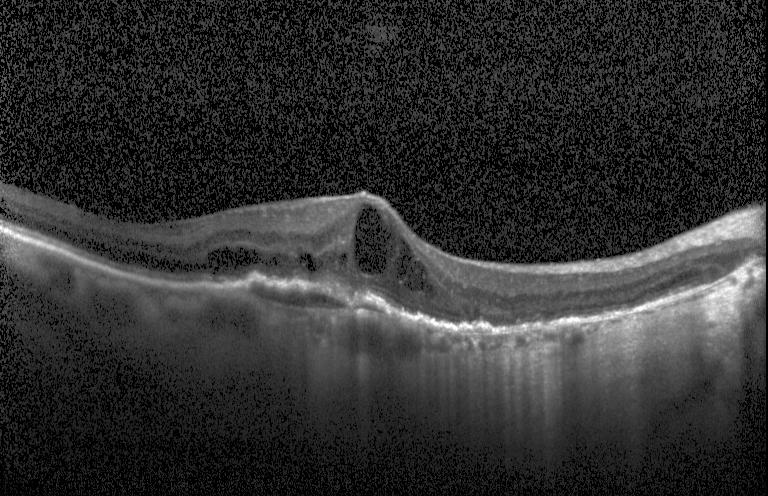 Diagnosis: CNV.